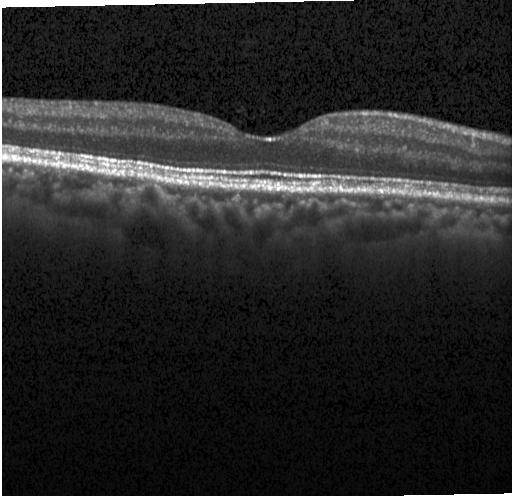

Retinal OCT cross-section showing no CNV, no DME, and no drusen.